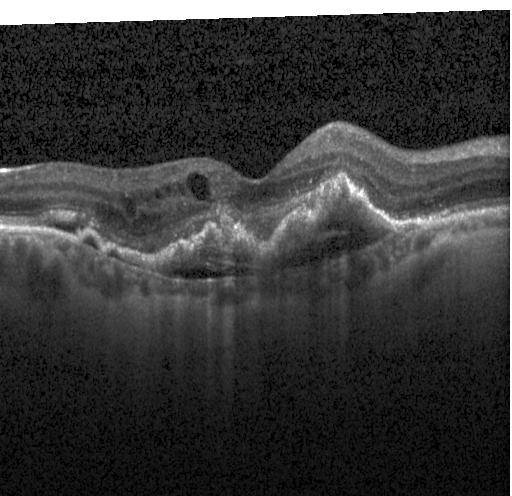
Assessment: CNV.